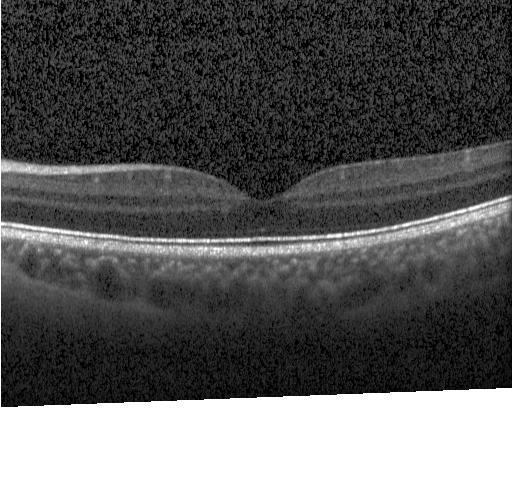
OCT line scan, instrument: Heidelberg Spectralis, spectral-domain optical coherence tomography
This B-scan demonstrates no choroidal neovascularization, no diabetic macular edema, and no drusen.